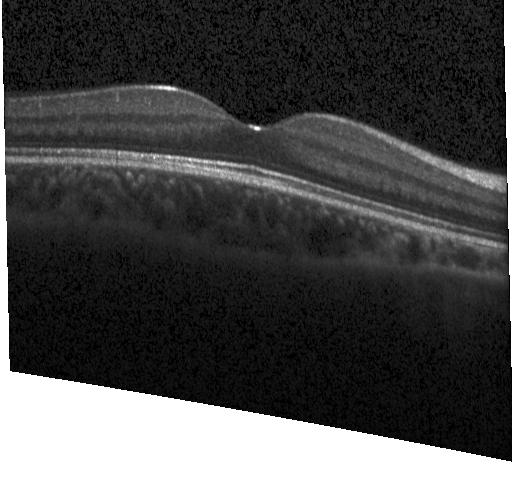

OCT line scan. SD-OCT
No choroidal neovascularization, diabetic macular edema, or drusen.